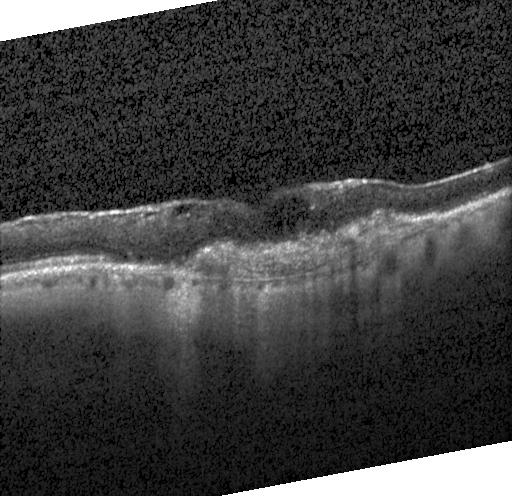 Optical coherence tomography B-scan · centered on the fovea · SD-OCT · acquired on a Heidelberg Spectralis.
Impression: CNV.